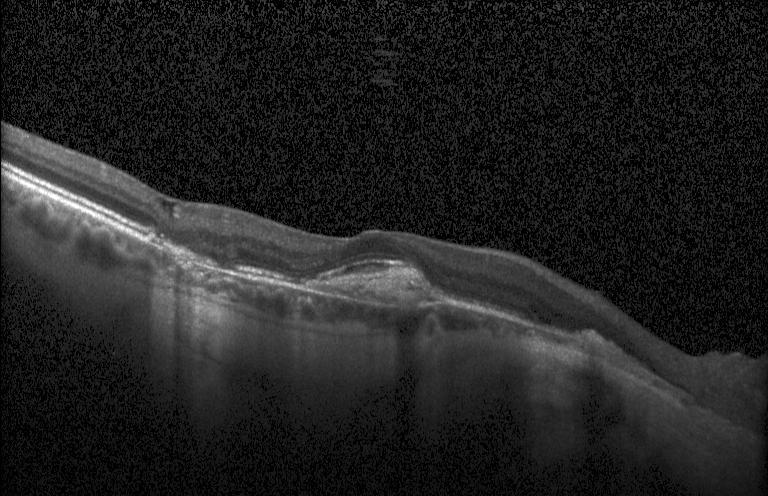

Macular scan · optical coherence tomography B-scan · acquired on a Heidelberg Spectralis — The scan shows choroidal neovascularization.